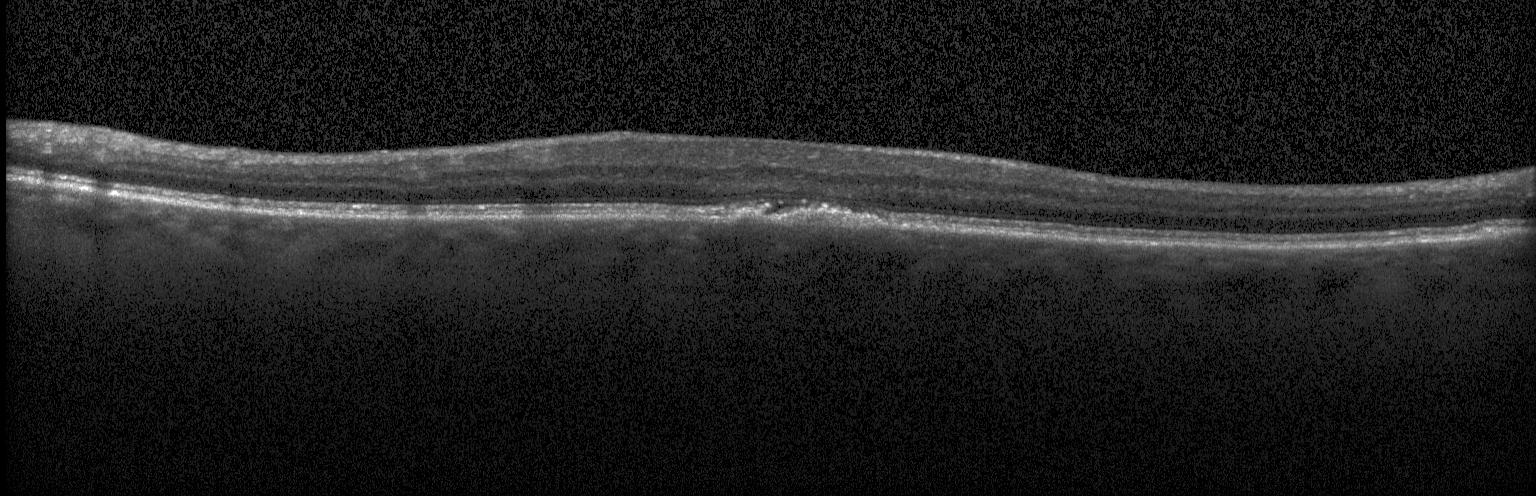
Retinal OCT cross-section. Heidelberg Spectralis OCT system — Finding: CNV.